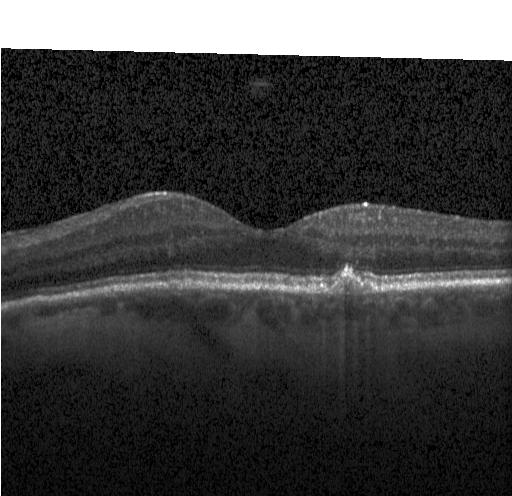

Finding: drusen.